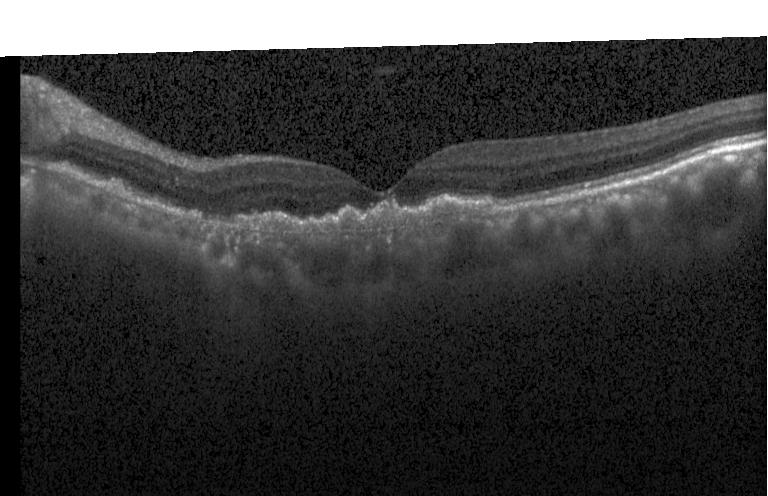
Horizontal scan through the fovea; retinal OCT cross-section — Diagnosis: a choroidal neovascular membrane.